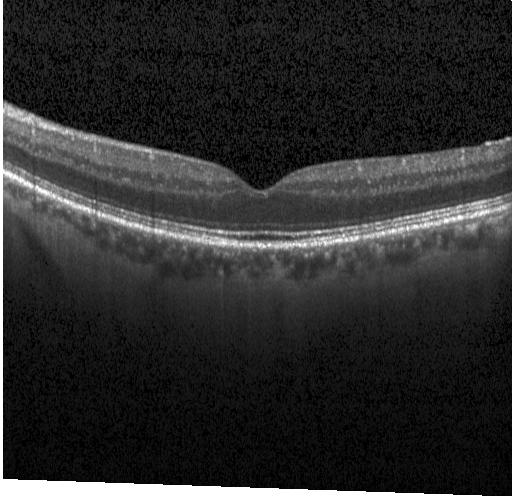

Spectral-domain optical coherence tomography. Horizontal scan through the fovea. Heidelberg Spectralis. Optical coherence tomography B-scan.
Finding: no choroidal neovascularization, diabetic macular edema, or drusen.